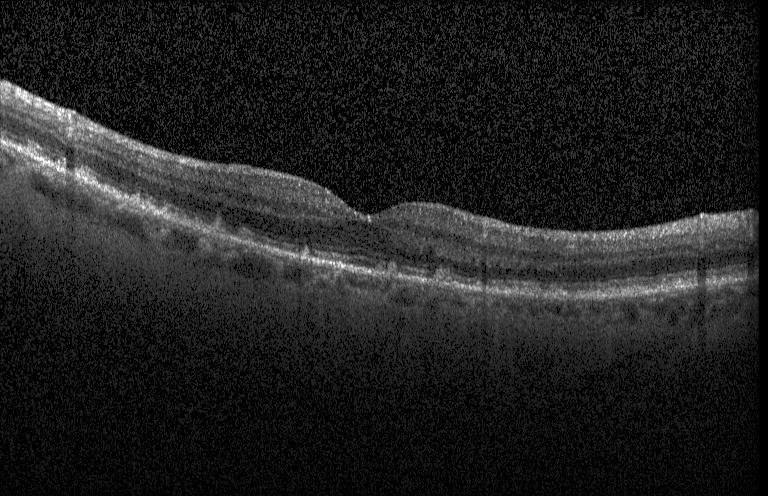 Retinal OCT cross-section; macular scan.
Assessment: drusen.